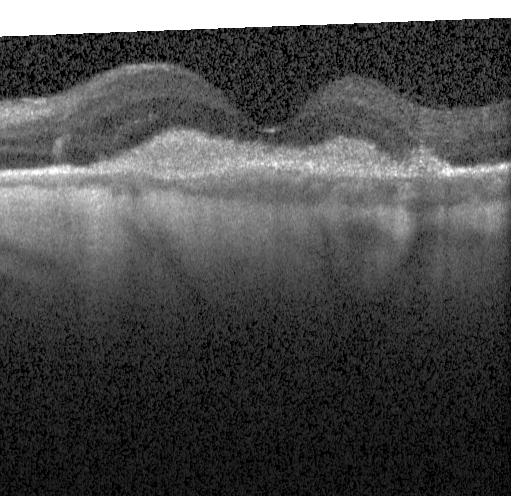 Macular scan; spectral-domain OCT; optical coherence tomography B-scan
A choroidal neovascular membrane.